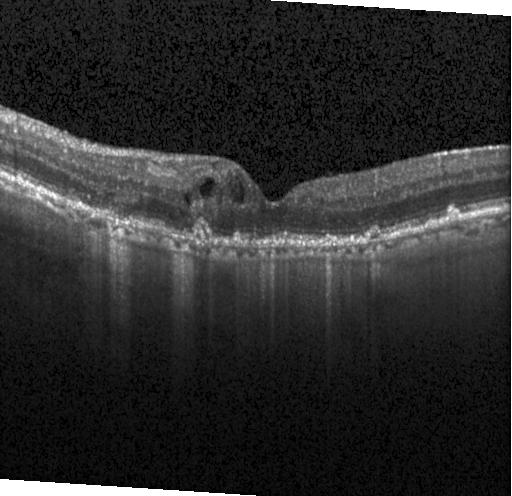
The scan shows choroidal neovascularization.